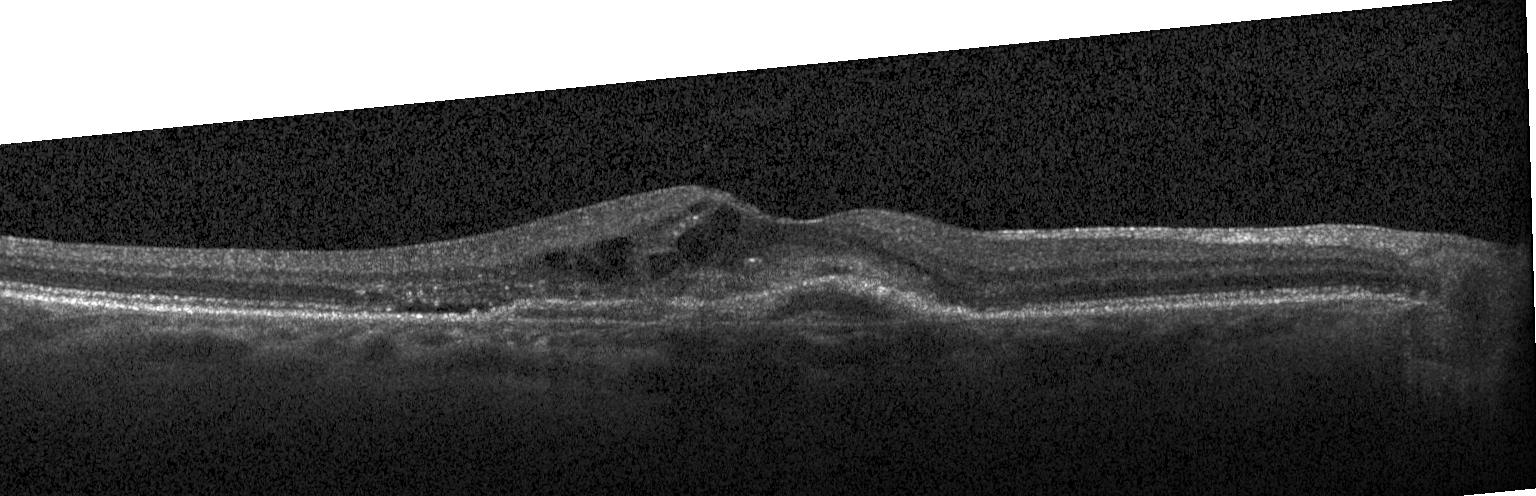

Spectral-domain OCT · horizontal scan through the fovea · OCT line scan — OCT finding: a choroidal neovascular membrane.